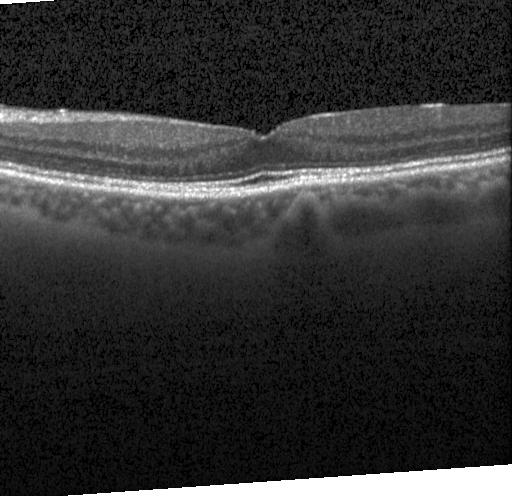

Finding: neither choroidal neovascularization, diabetic macular edema, nor drusen.